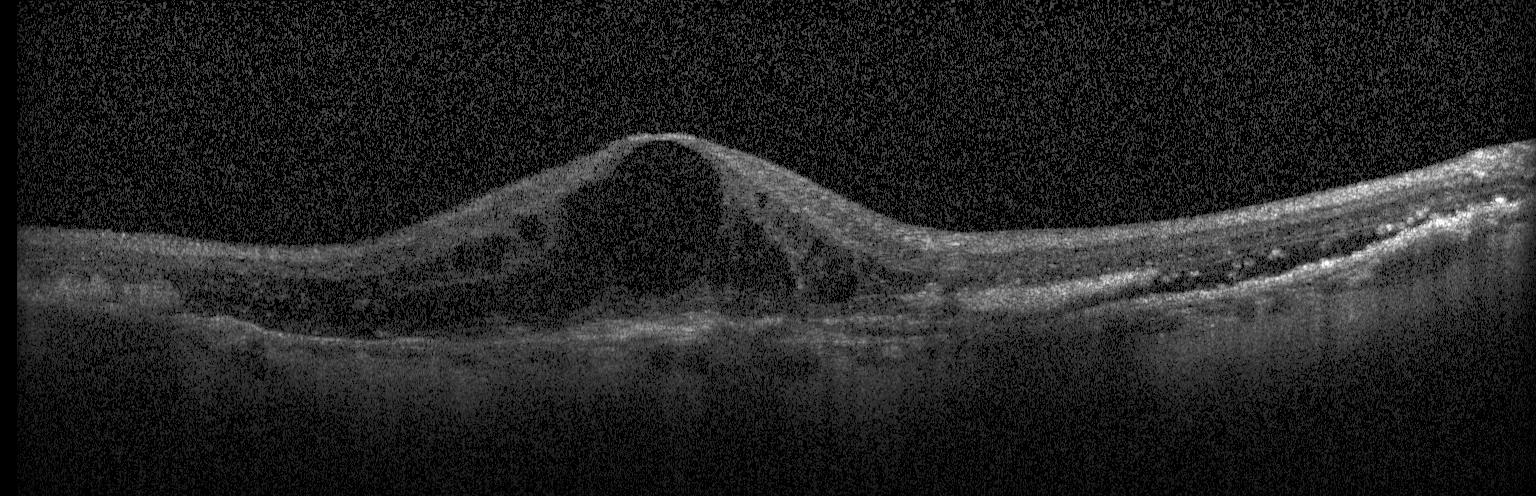 Dx: CNV.